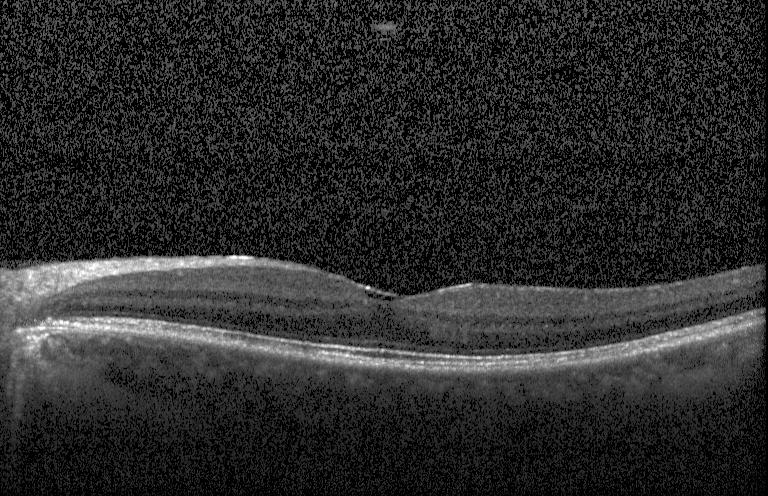 Acquired on a Heidelberg Spectralis, spectral-domain OCT, OCT B-scan.
Diagnosis: no CNV, DME, or drusen.